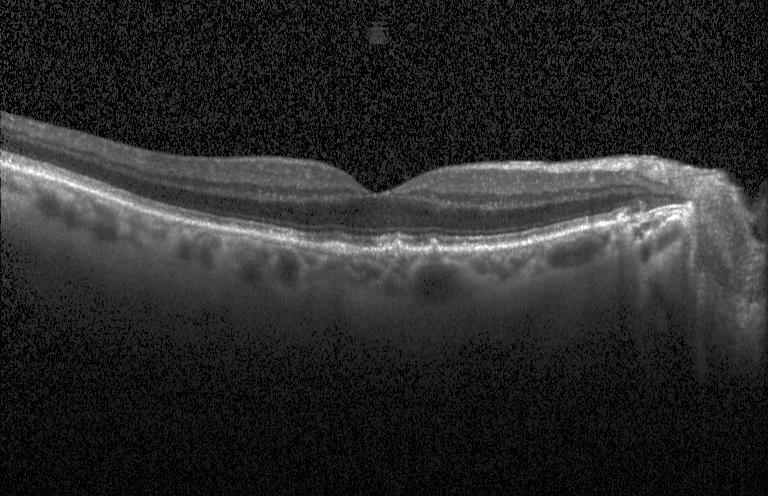 Dx: drusen.